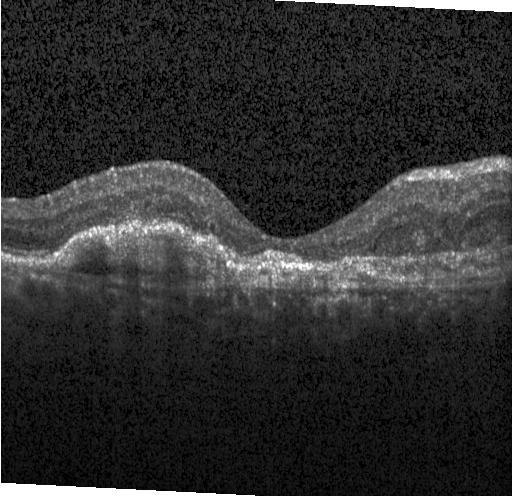

OCT B-scan
The scan shows a choroidal neovascular membrane.